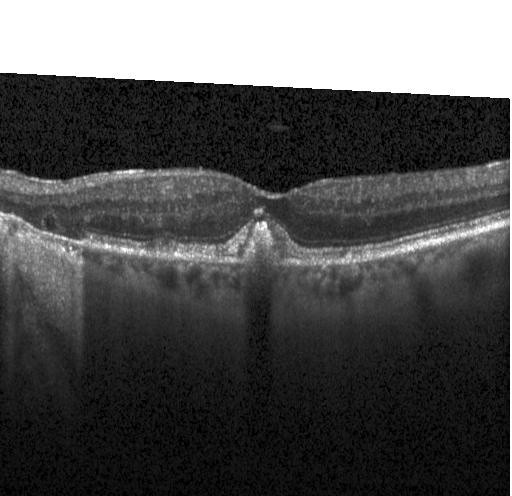

OCT finding: choroidal neovascularization.